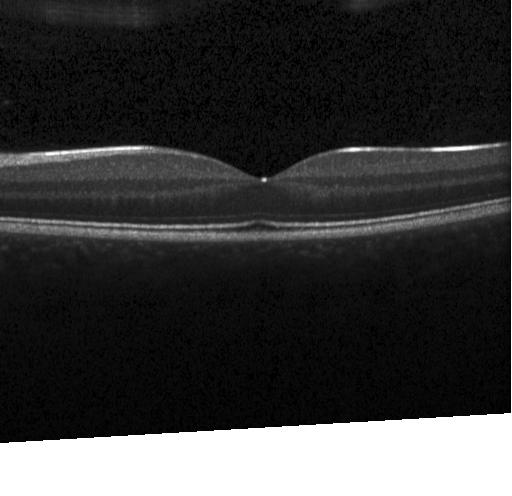 Spectral-domain optical coherence tomography, optical coherence tomography B-scan — Macular OCT: no choroidal neovascularization, diabetic macular edema, or drusen.